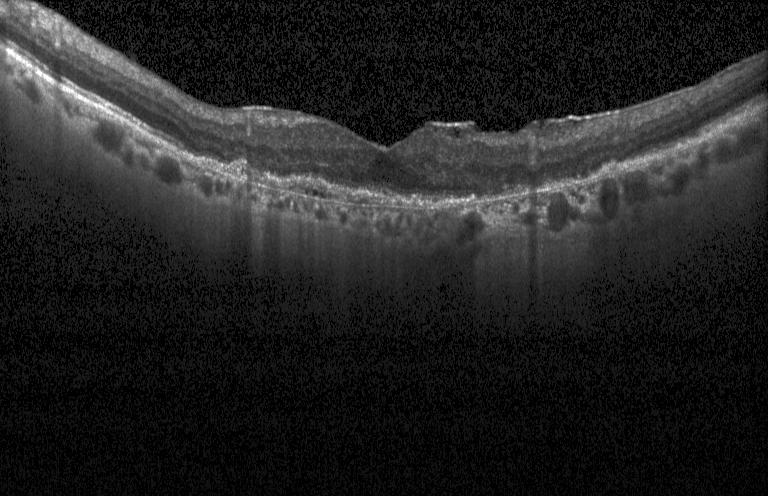
The scan shows a choroidal neovascular membrane.